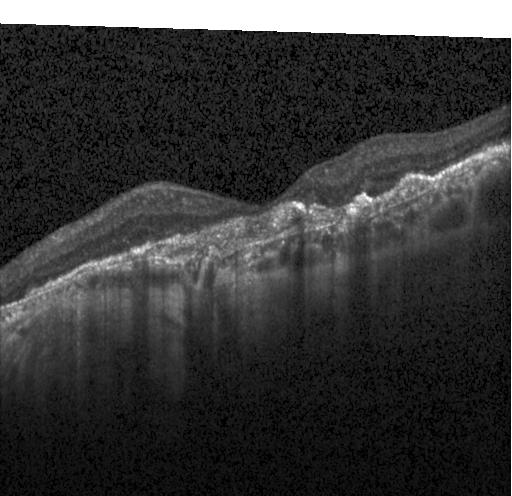

Optical coherence tomography B-scan. Heidelberg Spectralis
Impression: a choroidal neovascular membrane.